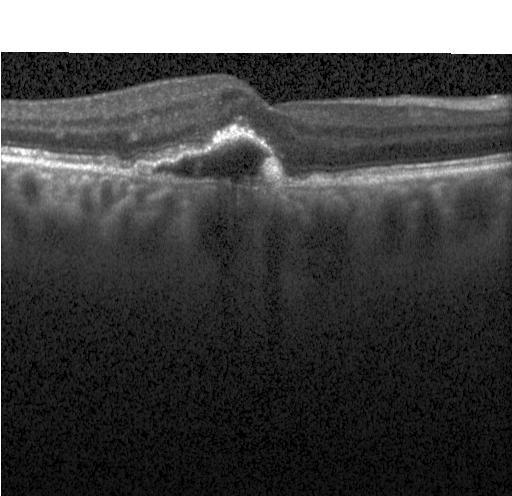 The scan shows a choroidal neovascular membrane.